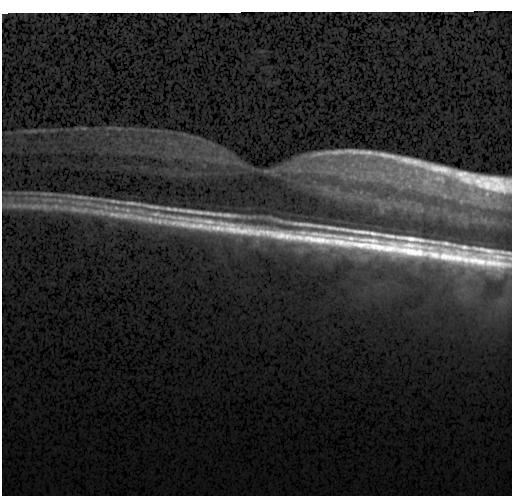
Retinal OCT B-scan — Diagnosis: no choroidal neovascularization, diabetic macular edema, or drusen.